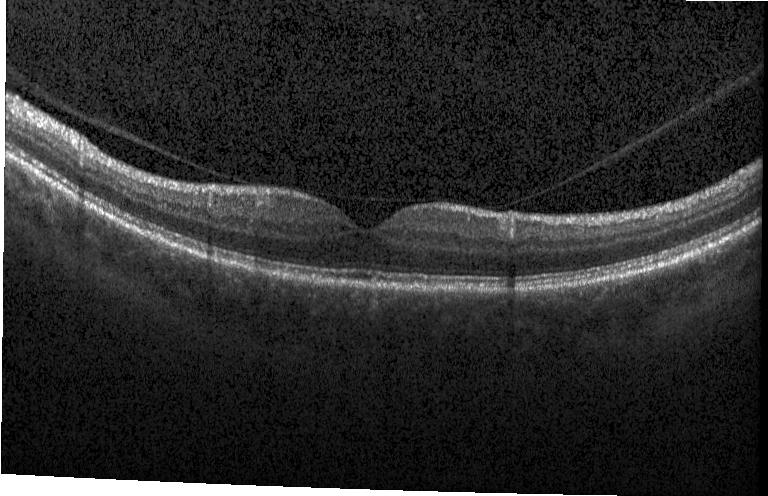
Acquired on a Heidelberg Spectralis. OCT B-scan. Neither CNV, DME, nor drusen.